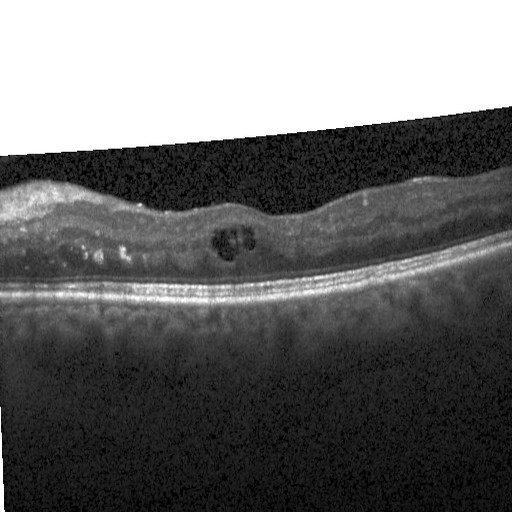

OCT line scan — Macular OCT: DME.